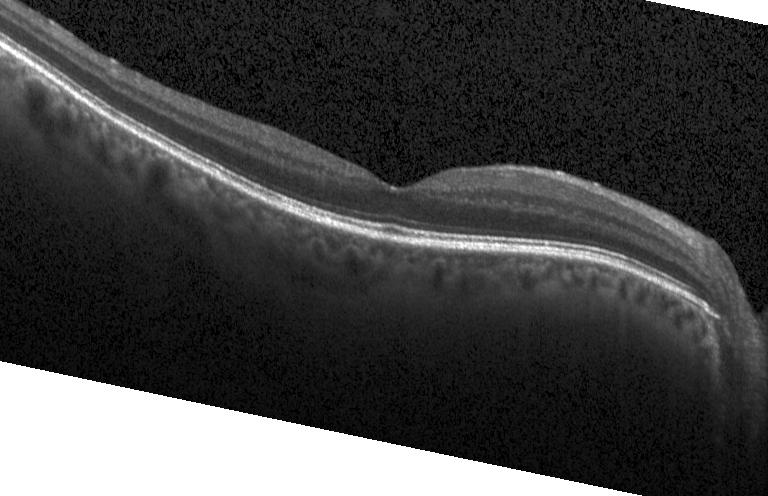 OCT B-scan showing no CNV, no DME, and no drusen.